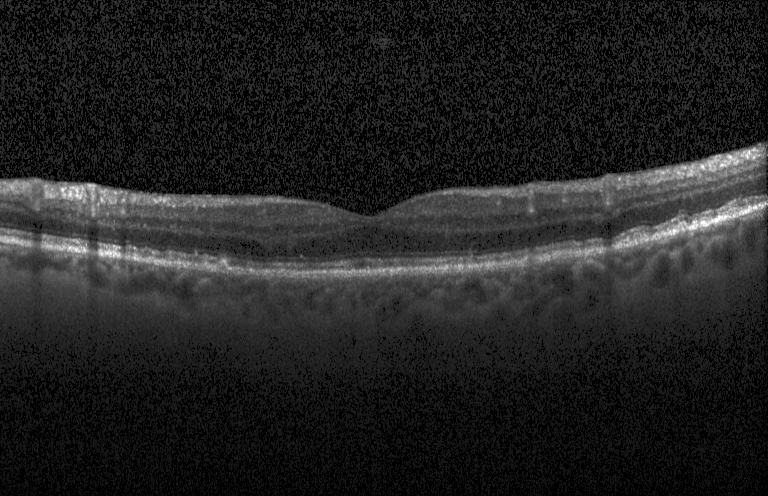

Finding: multiple drusen.